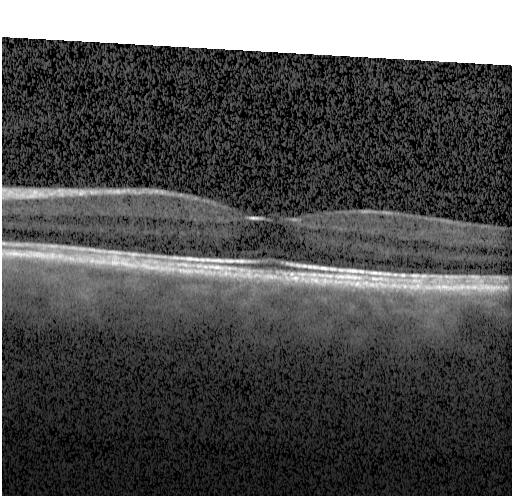

Macular OCT: no evidence of CNV, DME, or drusen.